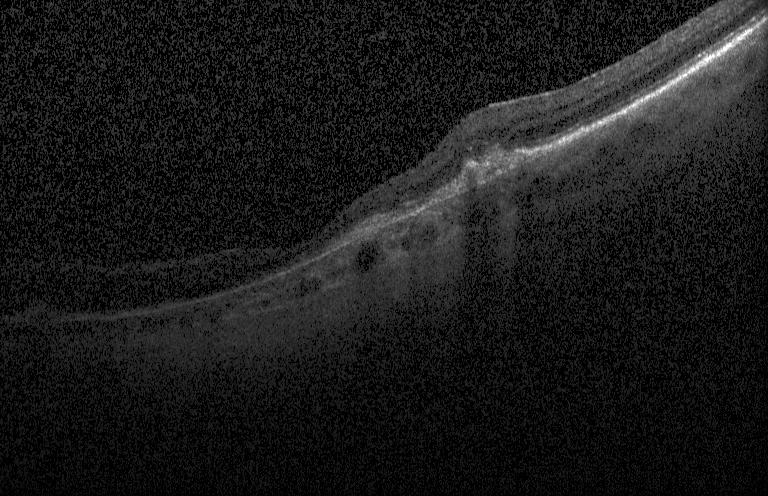
Retinal OCT B-scan — Diagnosis: choroidal neovascularization.